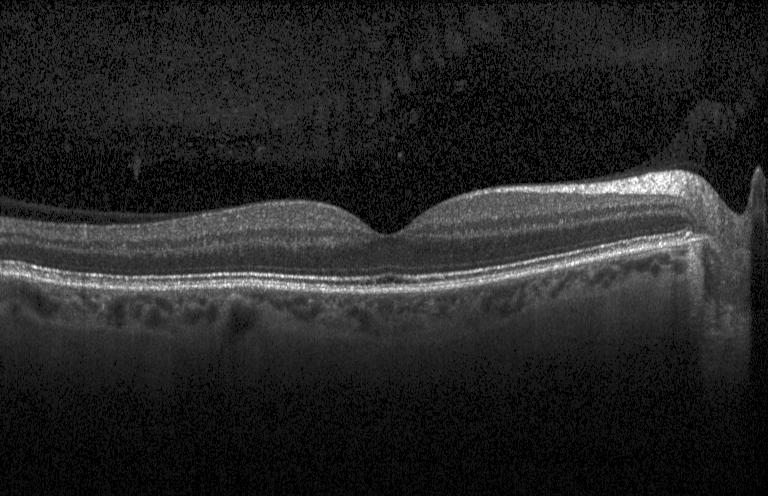
Optical coherence tomography B-scan, instrument: Heidelberg Spectralis — This B-scan demonstrates no choroidal neovascularization, diabetic macular edema, or drusen.